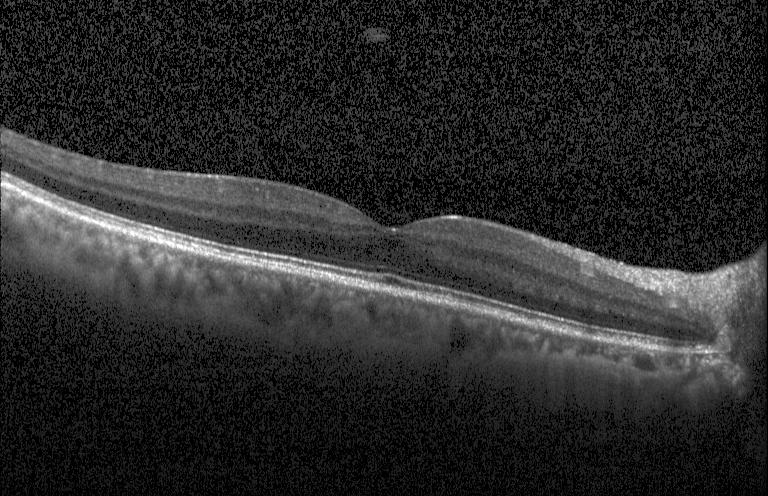
Centered on the fovea, Heidelberg Spectralis, spectral-domain optical coherence tomography, OCT B-scan. OCT finding: neither CNV, DME, nor drusen.